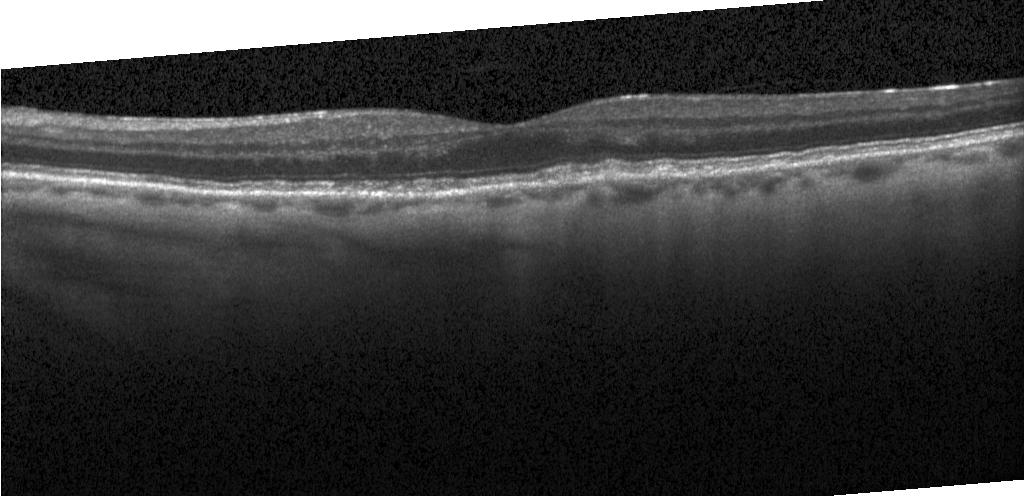
Retinal OCT cross-section; fovea-centered; spectral-domain optical coherence tomography; Heidelberg Spectralis. Impression: multiple drusen.